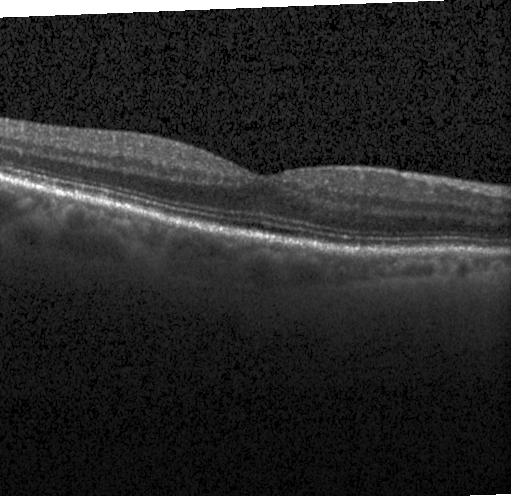 Centered on the fovea · spectral-domain OCT · acquired on a Heidelberg Spectralis · retinal OCT B-scan
Diagnosis: no choroidal neovascularization, no diabetic macular edema, and no drusen.